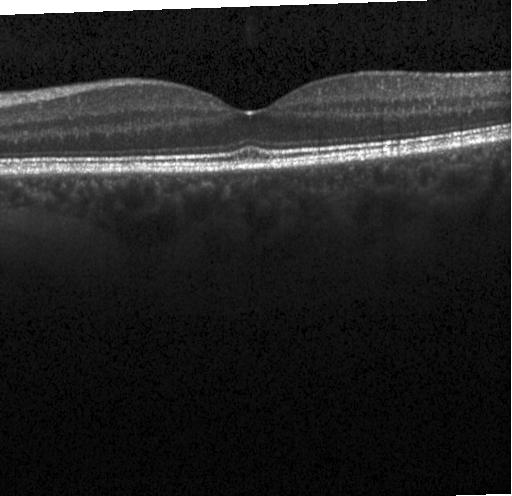

SD-OCT, Heidelberg Spectralis OCT system, optical coherence tomography scan.
The scan shows no evidence of CNV, DME, or drusen.